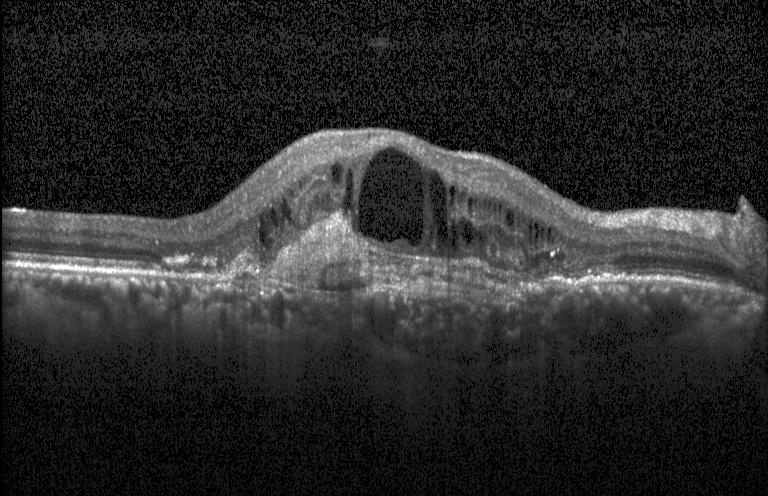

Retinal OCT B-scan.
A choroidal neovascular membrane.